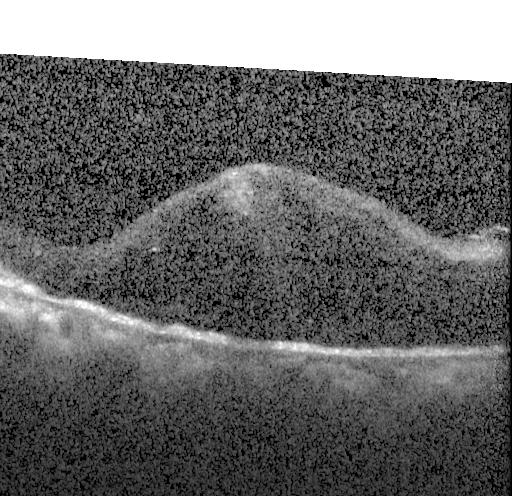 OCT scan showing DME.